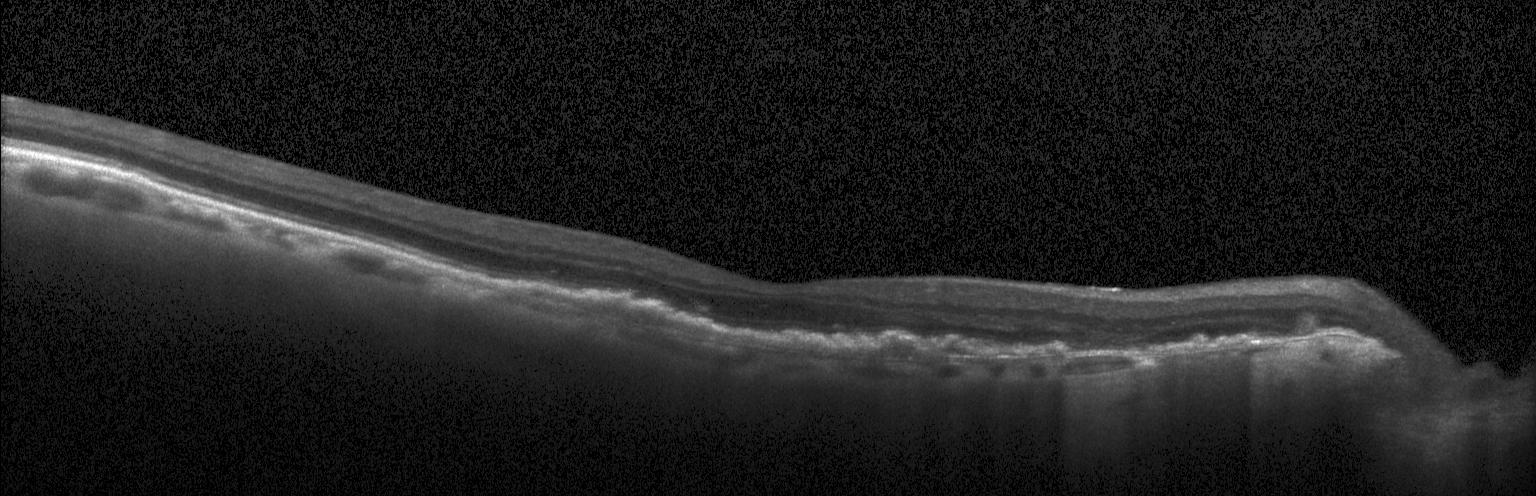 Dx: a choroidal neovascular membrane.